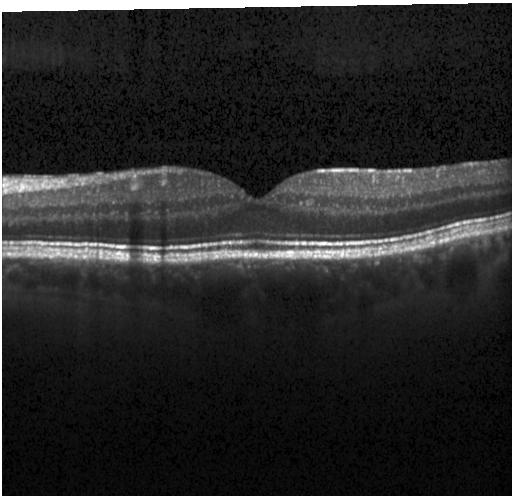

OCT line scan, spectral-domain optical coherence tomography — Macular OCT: no choroidal neovascularization, no diabetic macular edema, and no drusen.